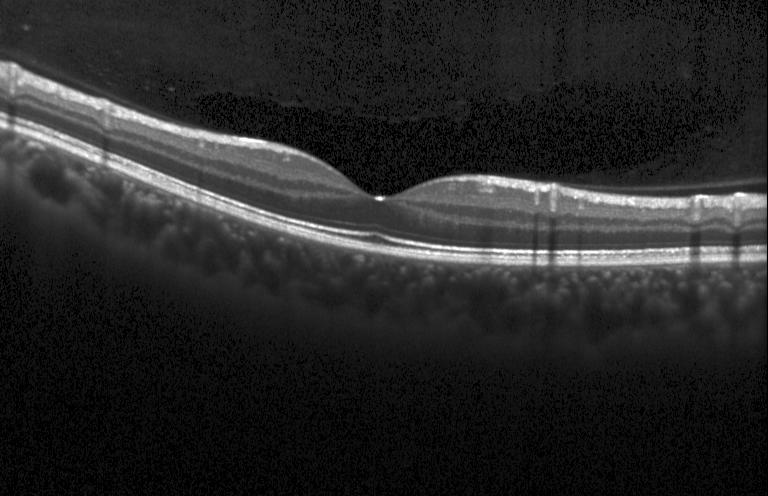

Spectral-domain OCT, OCT line scan
Assessment: no choroidal neovascularization, diabetic macular edema, or drusen.